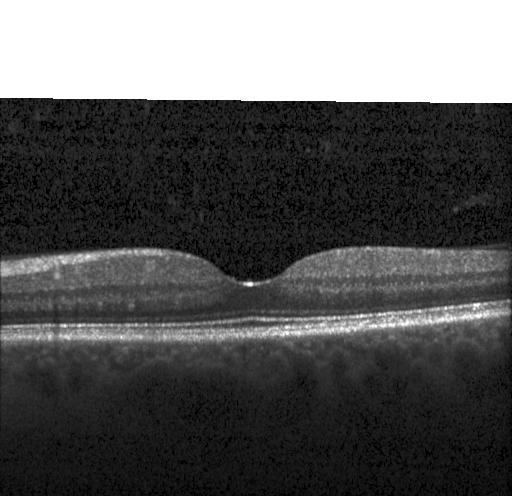

Impression: no evidence of choroidal neovascularization, diabetic macular edema, or drusen.